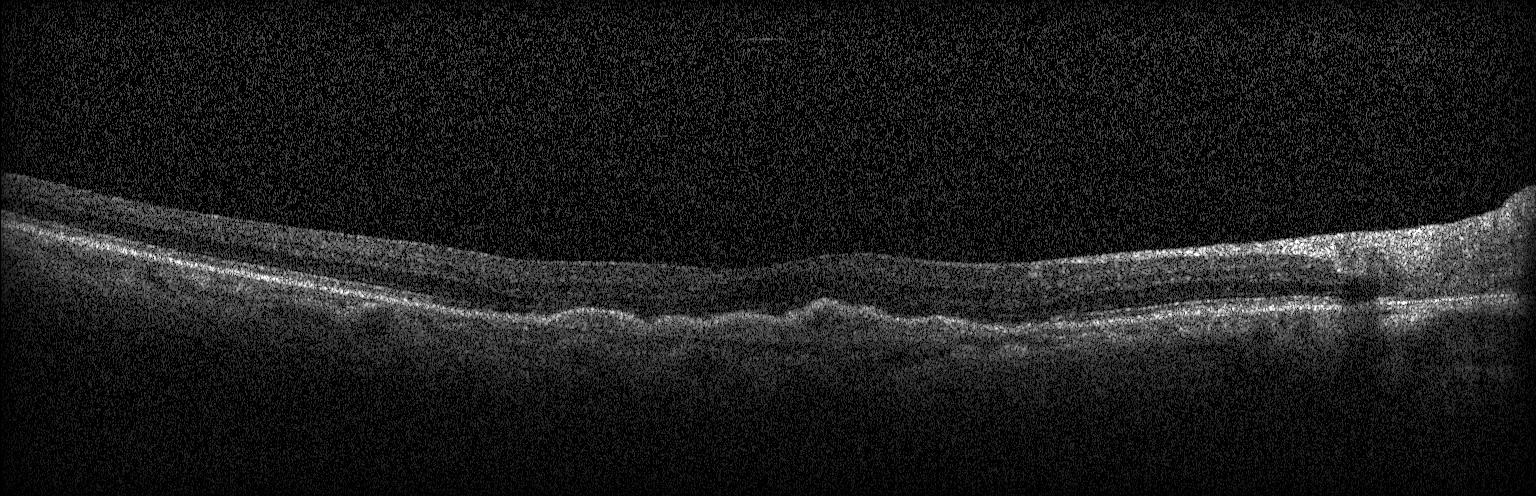 Optical coherence tomography B-scan · macular scan · spectral-domain OCT — Dx: a choroidal neovascular membrane.